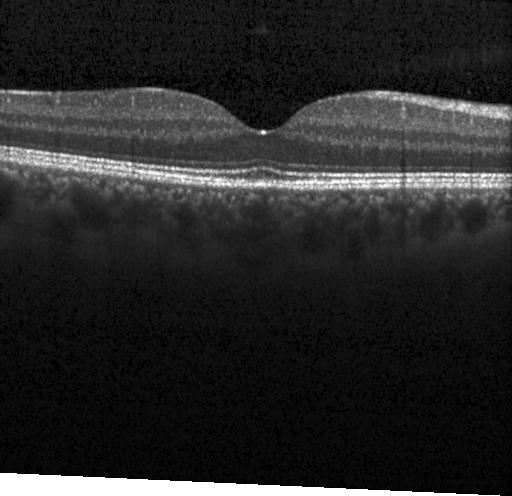

Optical coherence tomography scan.
OCT finding: no CNV, DME, or drusen.